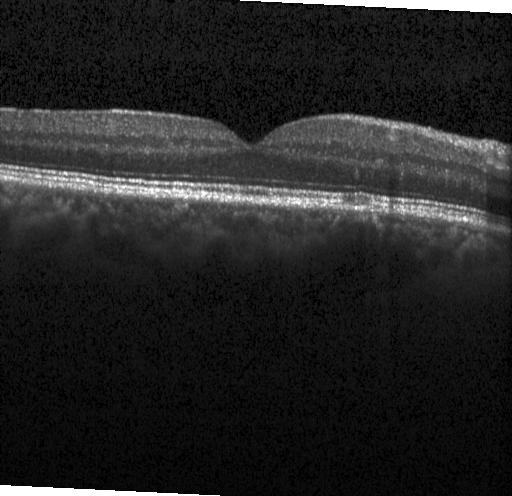 Retinal OCT cross-section
Finding: no choroidal neovascularization, diabetic macular edema, or drusen.